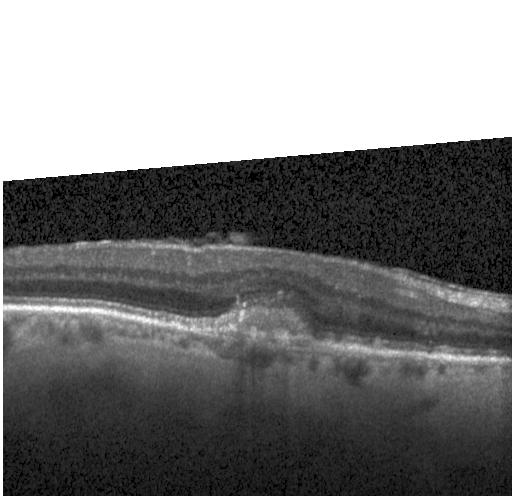
Heidelberg Spectralis, fovea-centered, retinal OCT B-scan, spectral-domain optical coherence tomography
Assessment: CNV.